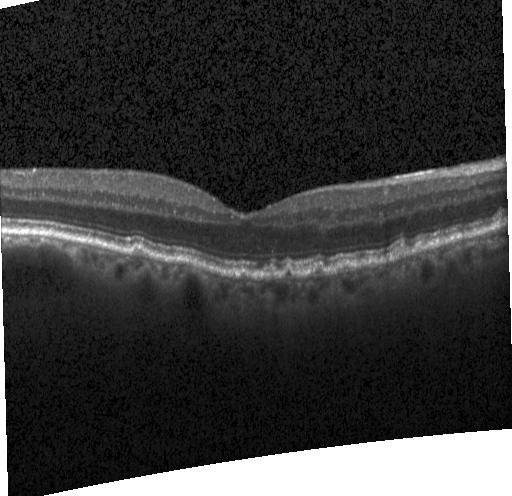 OCT finding: multiple drusen.